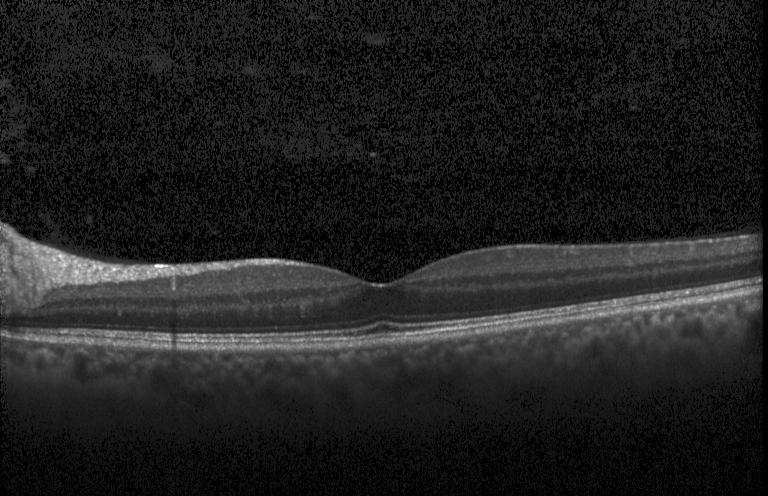
Spectral-domain OCT B-scan: no choroidal neovascularization, diabetic macular edema, or drusen.